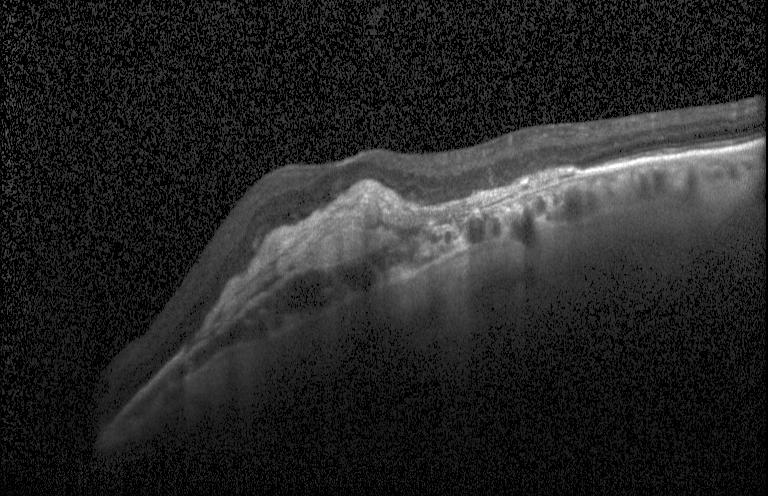 Optical coherence tomography B-scan; spectral-domain OCT
Impression: a choroidal neovascular membrane.